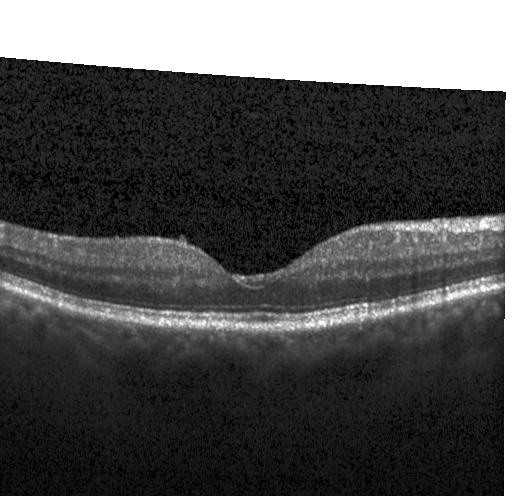

OCT B-scan. Spectral-domain optical coherence tomography — Dx: neither CNV, DME, nor drusen.